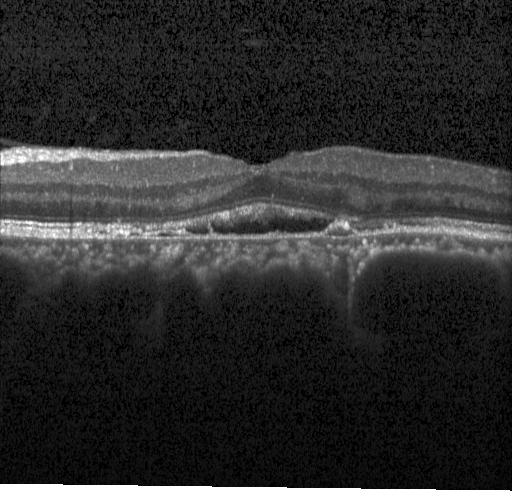

Fovea-centered, retinal OCT cross-section, acquired on a Heidelberg Spectralis. Impression: choroidal neovascularization (CNV).